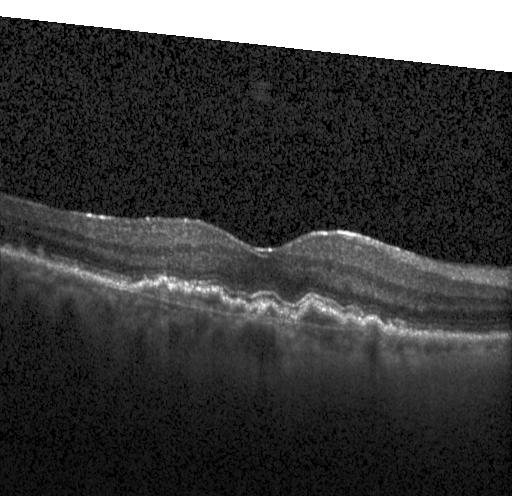

Retinal OCT B-scan
Dx: choroidal neovascularization (CNV).